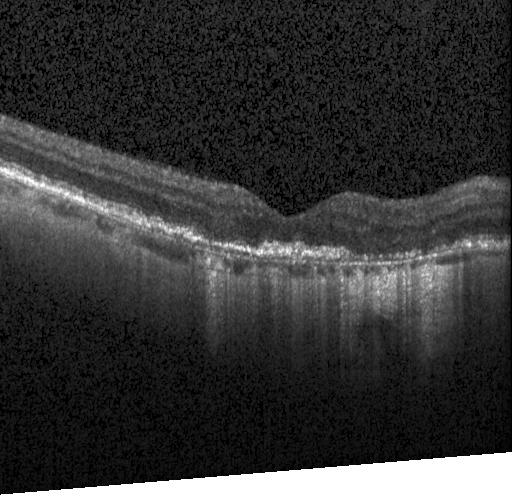
Heidelberg Spectralis. OCT B-scan
Macular OCT: CNV.